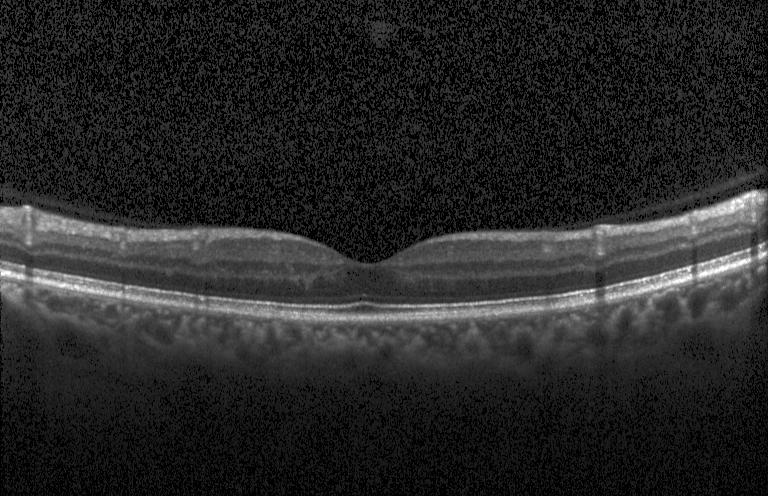
Macular OCT demonstrating no evidence of choroidal neovascularization, diabetic macular edema, or drusen.